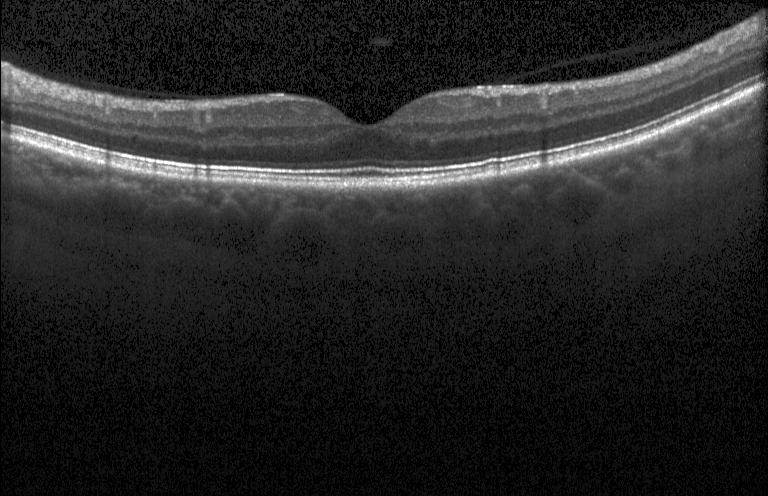
Dx: no choroidal neovascularization, no diabetic macular edema, and no drusen.